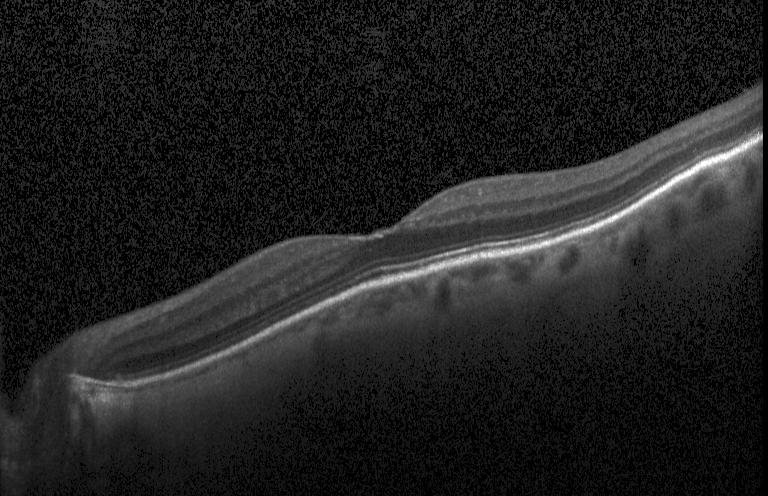 Finding: no choroidal neovascularization, diabetic macular edema, or drusen.